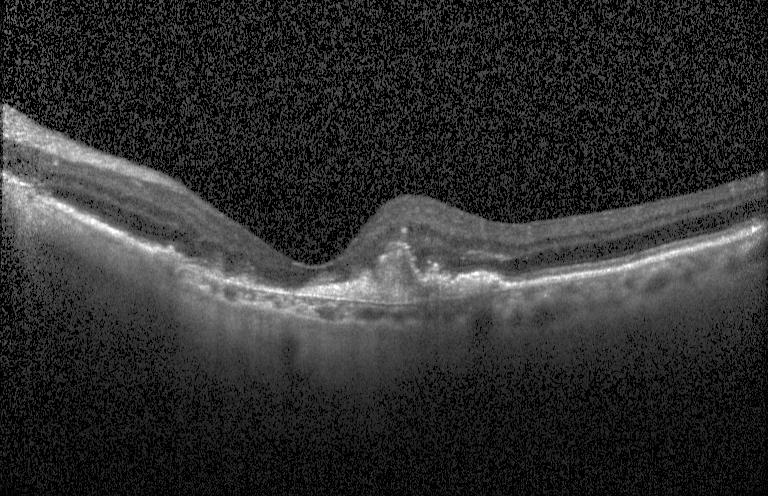
Macular OCT: choroidal neovascularization.